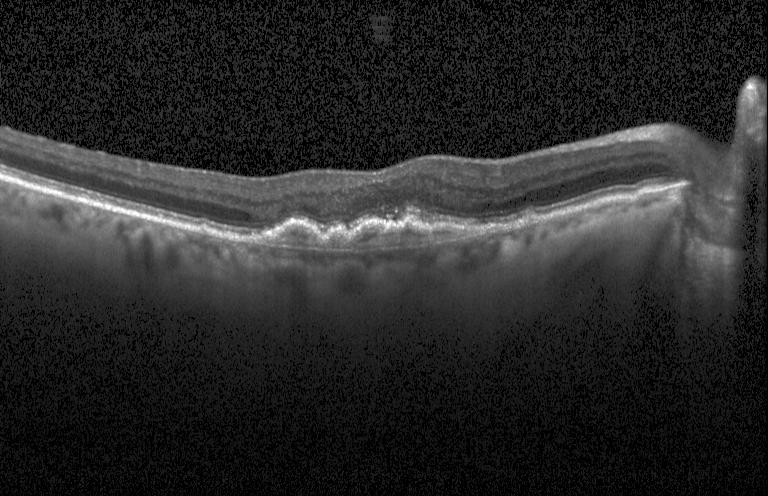 OCT B-scan; horizontal scan through the fovea; SD-OCT — A choroidal neovascular membrane.